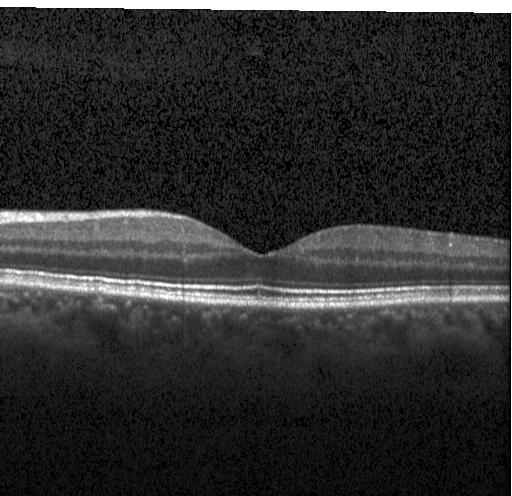

Diagnosis: neither choroidal neovascularization, diabetic macular edema, nor drusen.